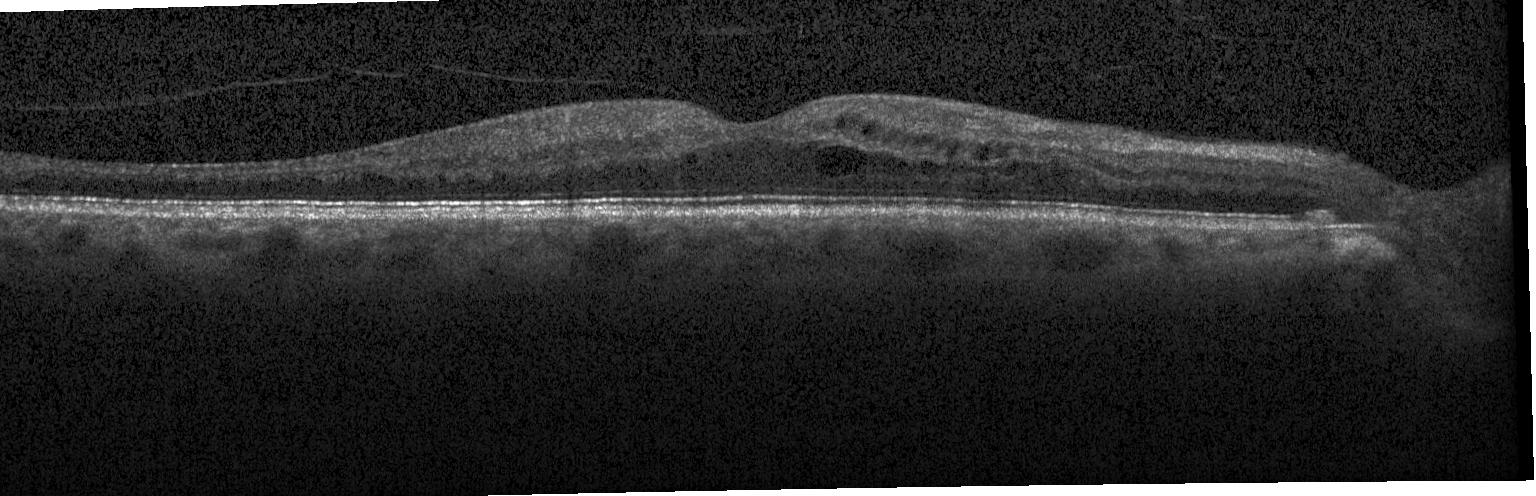
Heidelberg Spectralis OCT system · fovea-centered · retinal OCT cross-section.
The scan shows DME.